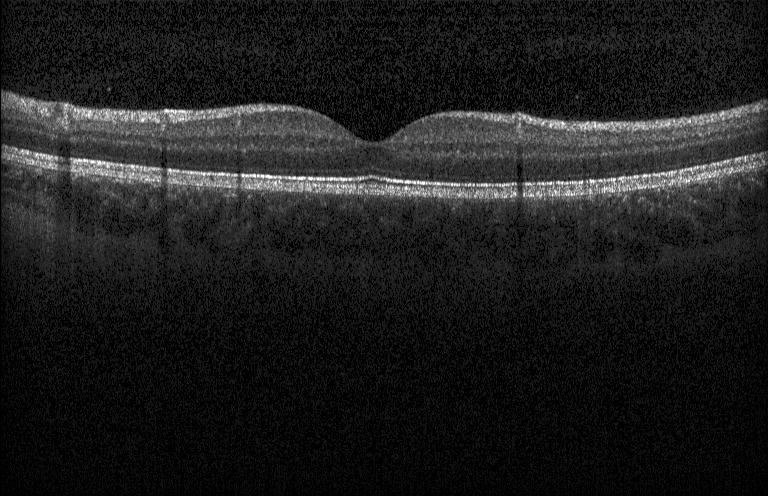

Spectral-domain optical coherence tomography, instrument: Heidelberg Spectralis, optical coherence tomography scan
Assessment: no evidence of choroidal neovascularization, diabetic macular edema, or drusen.